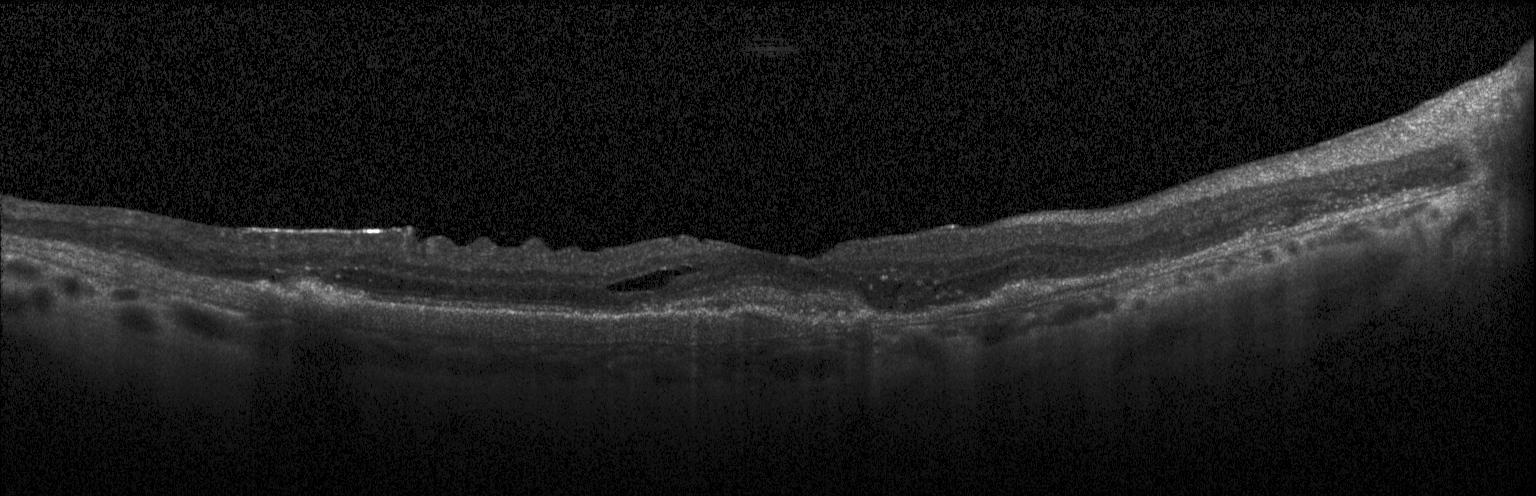
SD-OCT; fovea-centered; retinal OCT cross-section; Heidelberg Spectralis OCT system
This B-scan demonstrates a choroidal neovascular membrane.